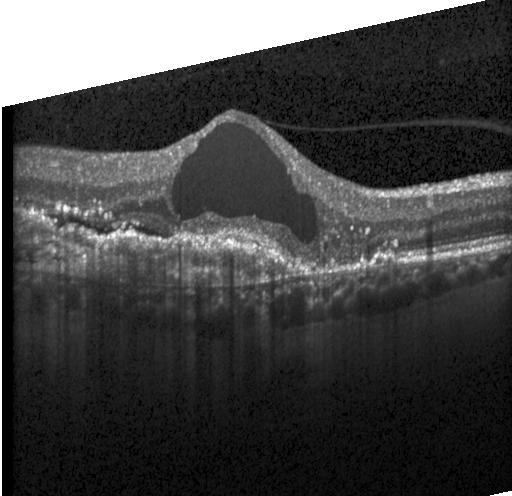 Through the macula; optical coherence tomography B-scan; Heidelberg Spectralis
Dx: a choroidal neovascular membrane.